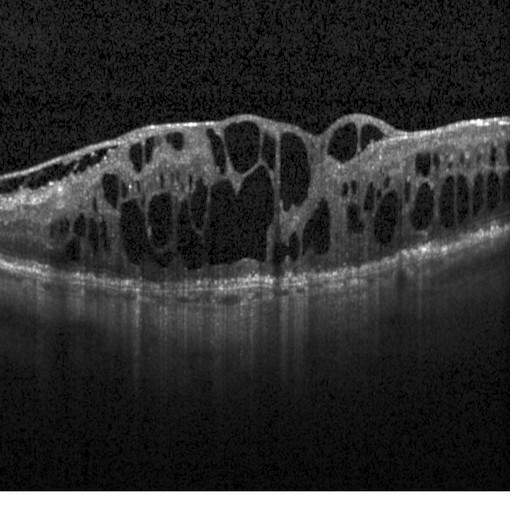

Centered on the fovea · OCT line scan · Heidelberg Spectralis · spectral-domain optical coherence tomography.
Diagnosis: diabetic macular edema.